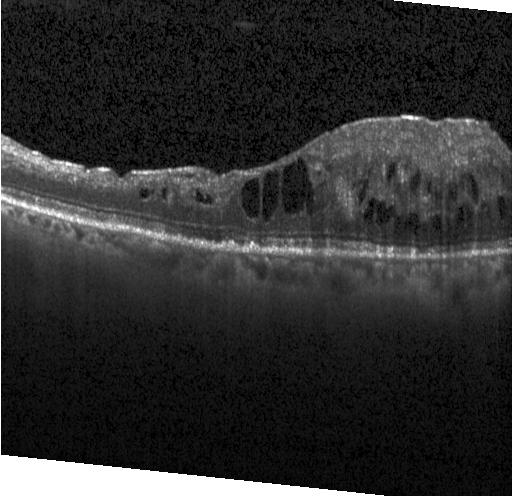 This B-scan demonstrates diabetic macular edema (DME).